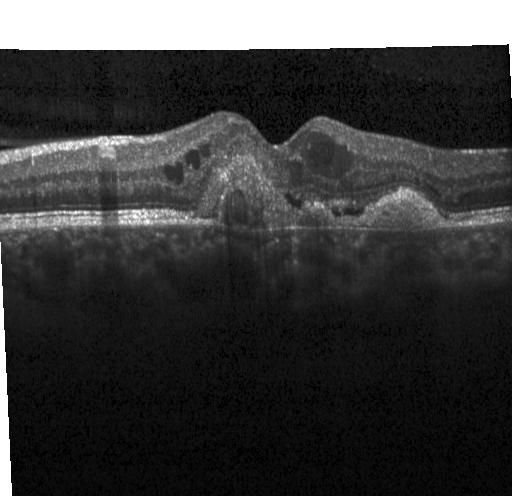
Retinal OCT cross-section showing choroidal neovascularization (CNV).